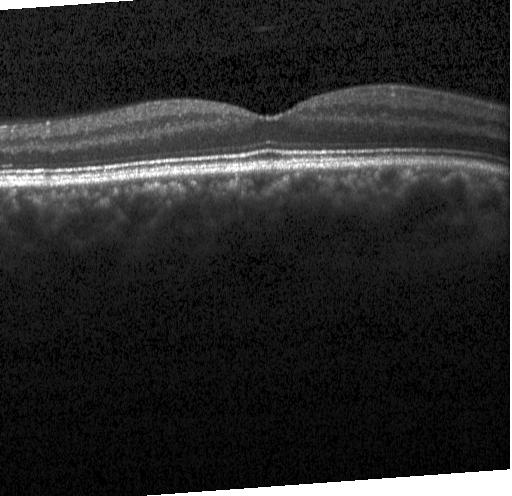
No evidence of choroidal neovascularization, diabetic macular edema, or drusen.